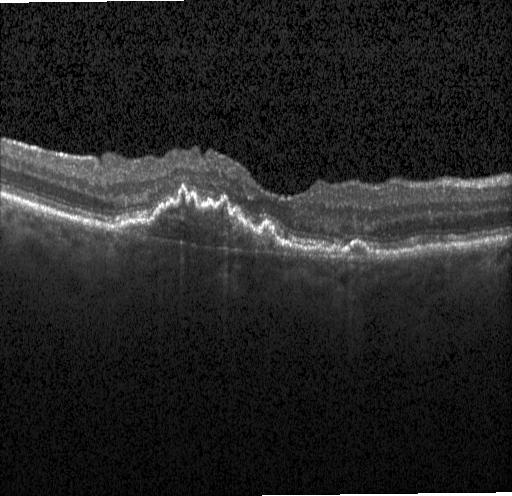 Spectral-domain OCT · instrument: Heidelberg Spectralis · retinal OCT B-scan · horizontal scan through the fovea
Finding: CNV.